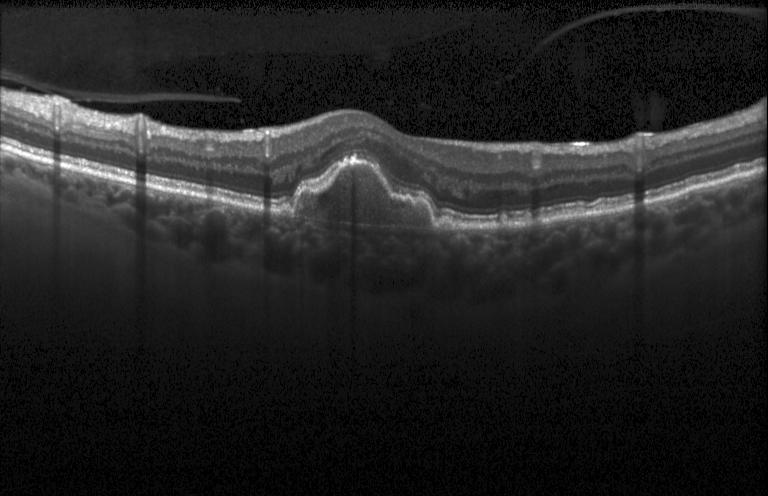 SD-OCT, retinal OCT B-scan.
Impression: choroidal neovascularization (CNV).